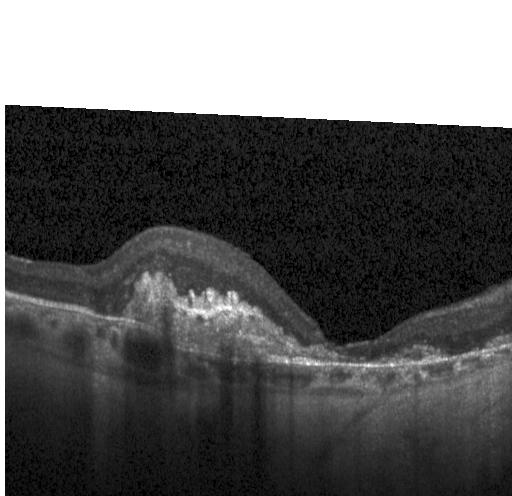

Finding: a choroidal neovascular membrane.